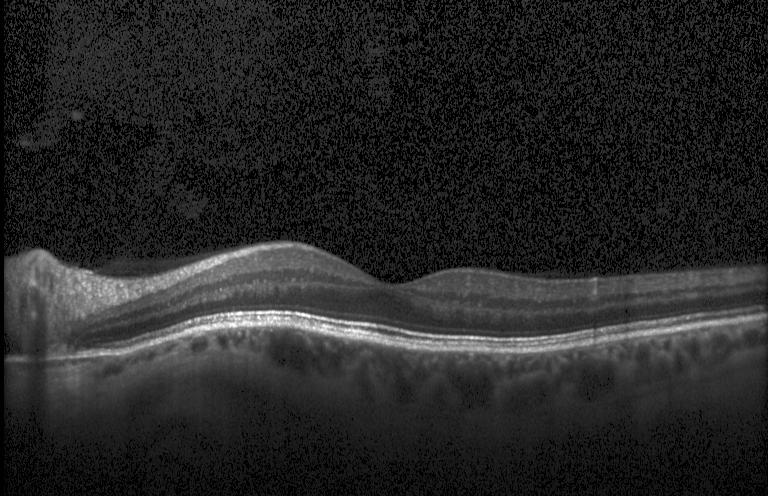

SD-OCT · retinal OCT cross-section · Heidelberg Spectralis · through the macula.
Macular OCT: no choroidal neovascularization, diabetic macular edema, or drusen.